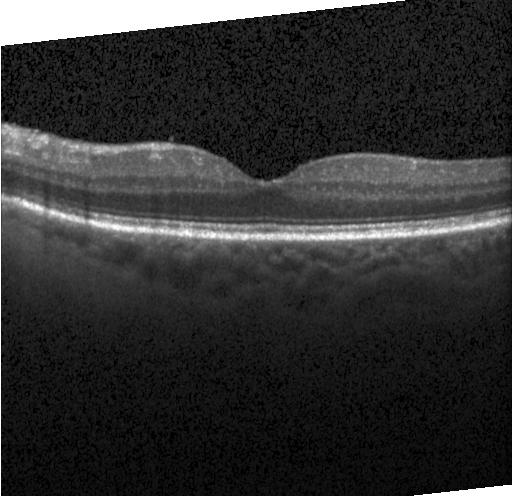 Retinal OCT cross-section · Heidelberg Spectralis.
Diagnosis: no CNV, no DME, and no drusen.